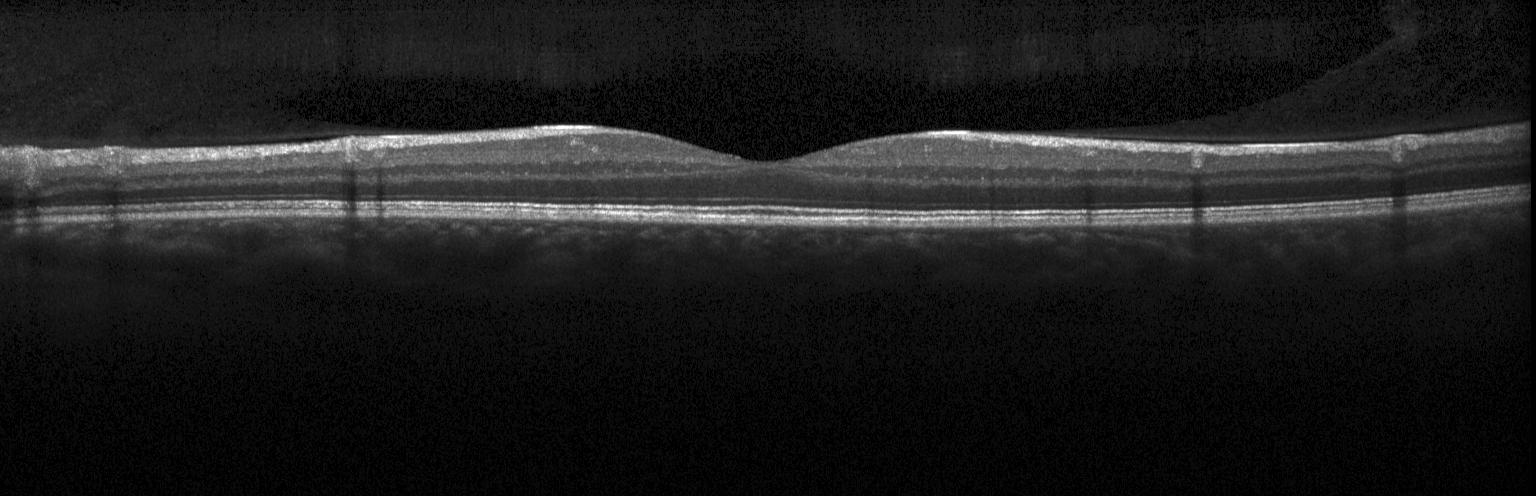 Spectral-domain OCT. Optical coherence tomography scan. Centered on the fovea. Acquired on a Heidelberg Spectralis — No evidence of choroidal neovascularization, diabetic macular edema, or drusen.